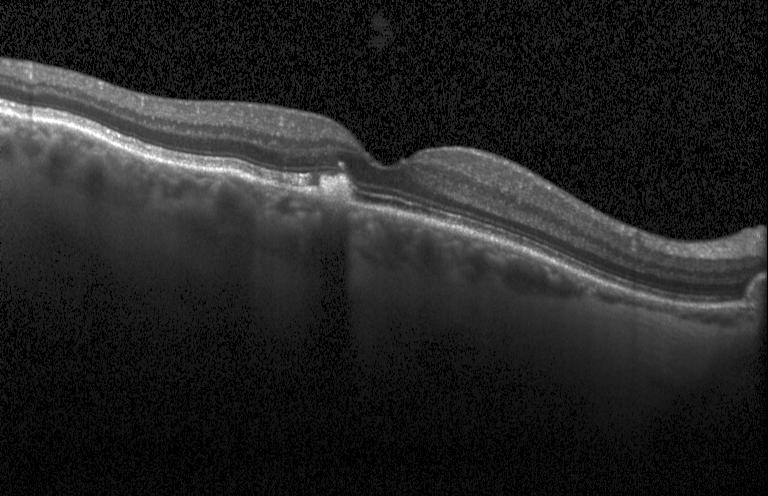

SD-OCT. Optical coherence tomography B-scan. Fovea-centered. Finding: multiple drusen.